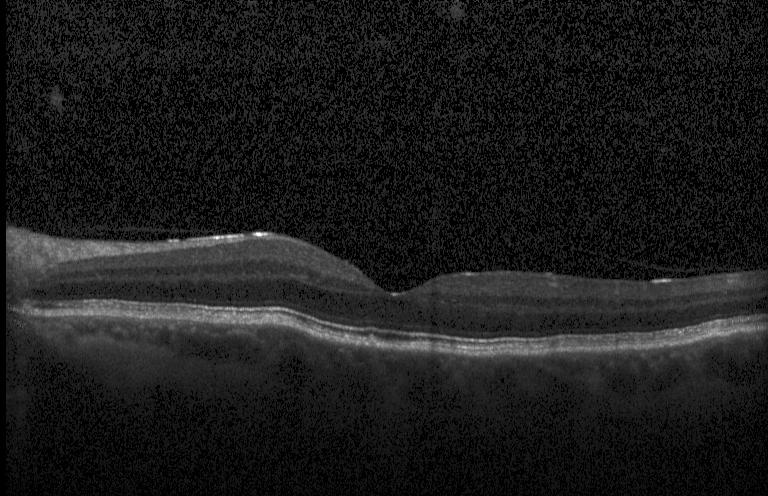 Instrument: Heidelberg Spectralis, horizontal scan through the fovea, OCT line scan, spectral-domain optical coherence tomography
Finding: no choroidal neovascularization, no diabetic macular edema, and no drusen.